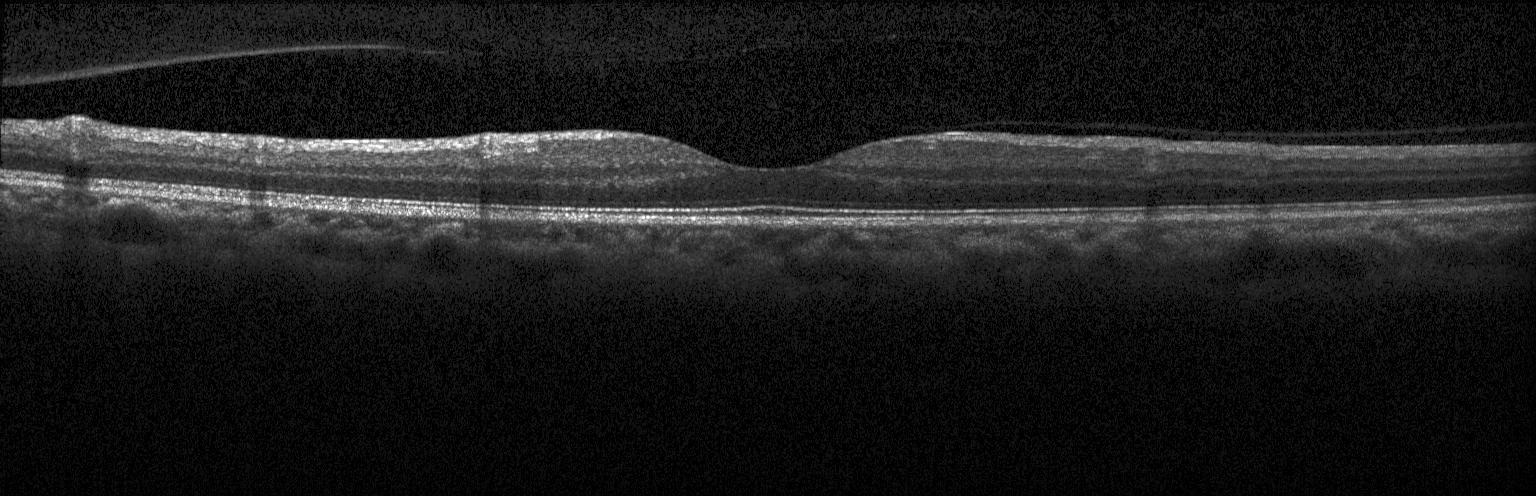 SD-OCT; retinal OCT cross-section. OCT finding: neither CNV, DME, nor drusen.